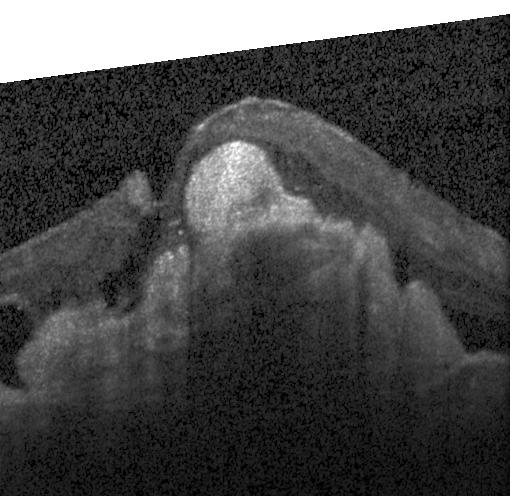

Centered on the fovea. Acquired on a Heidelberg Spectralis. Optical coherence tomography B-scan — Finding: a choroidal neovascular membrane.